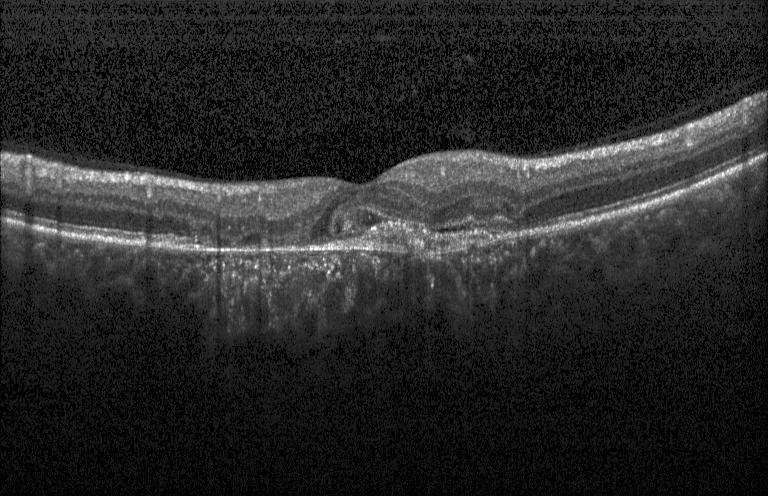
Macular scan, SD-OCT, OCT line scan, instrument: Heidelberg Spectralis. Finding: a choroidal neovascular membrane.